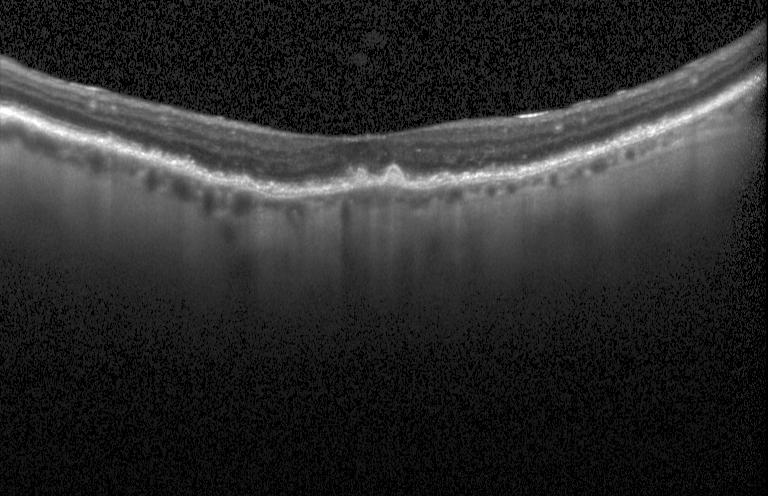
Acquired on a Heidelberg Spectralis · OCT B-scan
Assessment: a choroidal neovascular membrane.